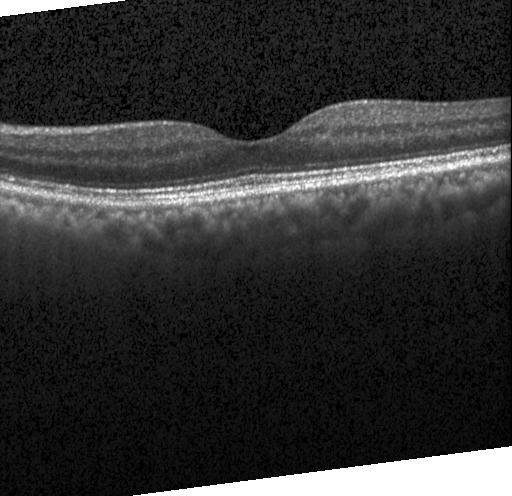

OCT line scan
Diagnosis: neither choroidal neovascularization, diabetic macular edema, nor drusen.